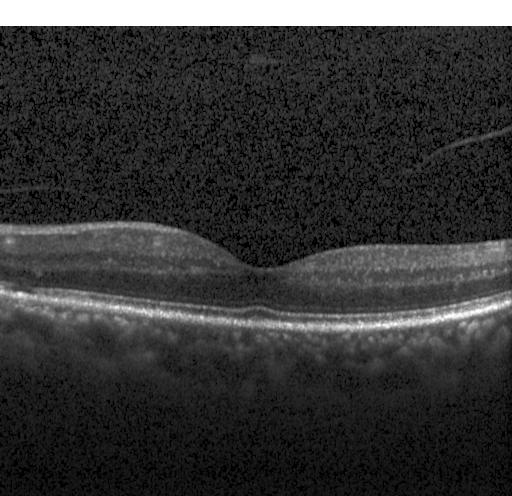
OCT line scan.
No CNV, DME, or drusen.